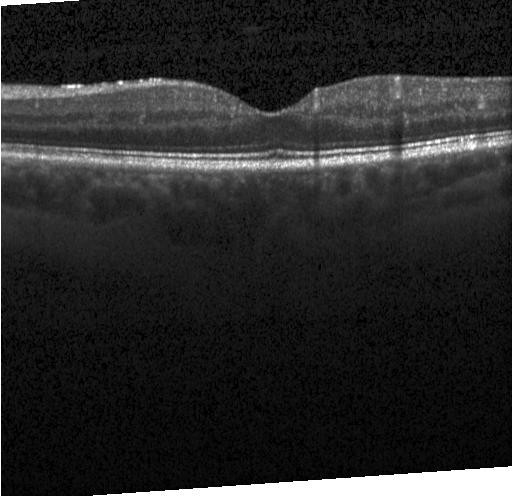

OCT scan showing no evidence of CNV, DME, or drusen.